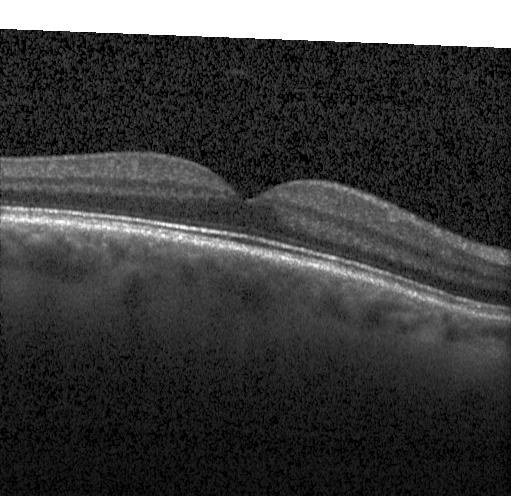 This B-scan demonstrates no choroidal neovascularization, diabetic macular edema, or drusen.